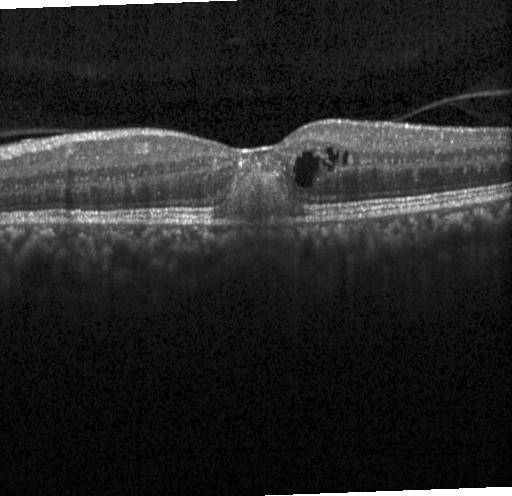
Horizontal scan through the fovea. Retinal OCT cross-section. SD-OCT. Assessment: a choroidal neovascular membrane.